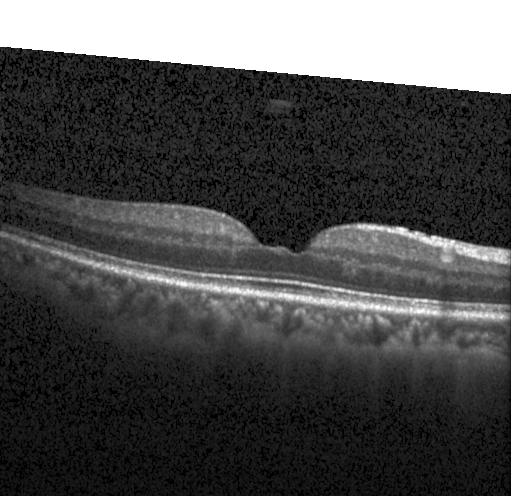

Dx: neither choroidal neovascularization, diabetic macular edema, nor drusen.